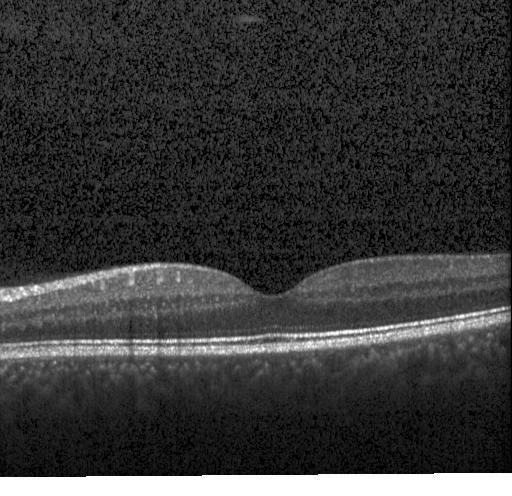

Dx: neither CNV, DME, nor drusen.